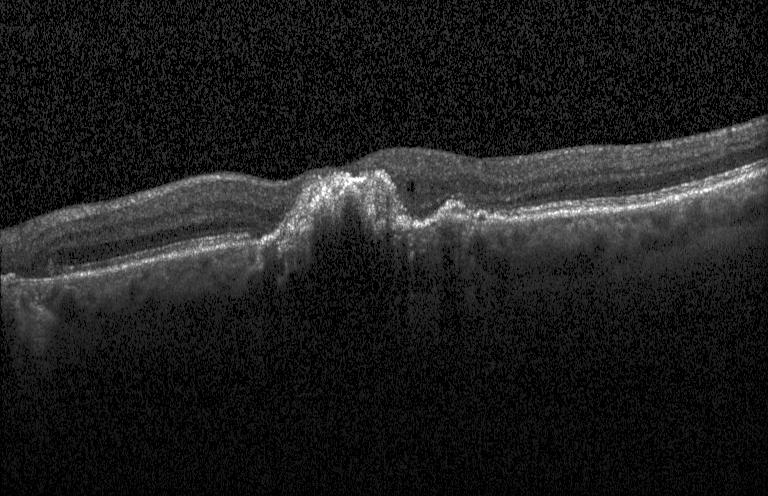 Acquired on a Heidelberg Spectralis; optical coherence tomography B-scan. Diagnosis: a choroidal neovascular membrane.